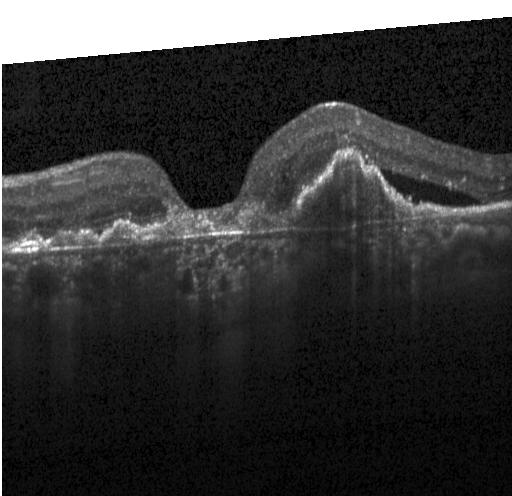
Horizontal scan through the fovea. Optical coherence tomography scan. OCT finding: choroidal neovascularization (CNV).